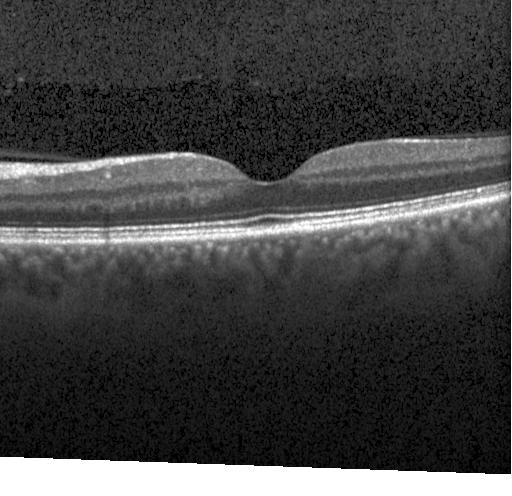

Spectral-domain OCT; retinal OCT cross-section. Dx: neither choroidal neovascularization, diabetic macular edema, nor drusen.